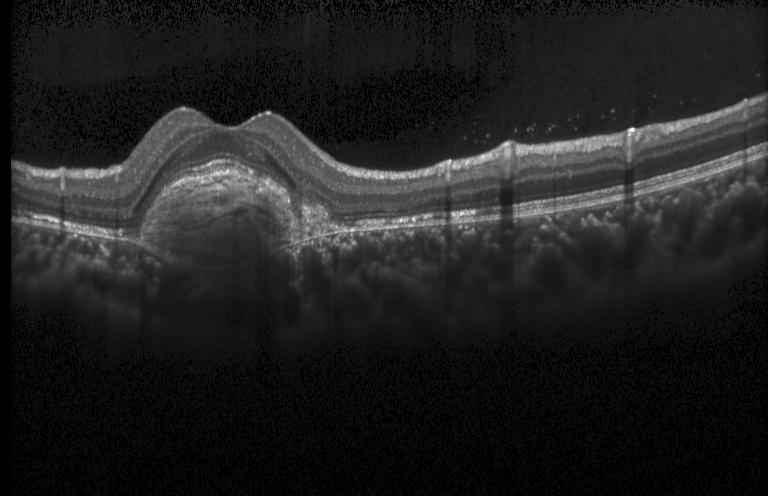
Retinal OCT cross-section, through the macula — Impression: CNV.